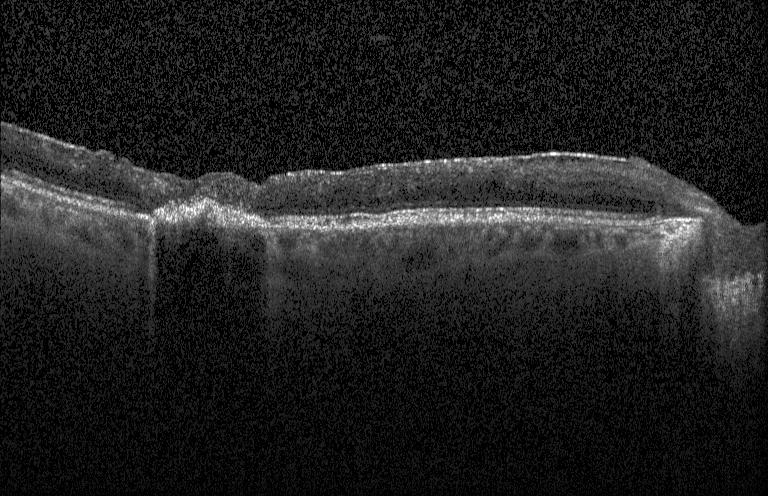 OCT line scan. Instrument: Heidelberg Spectralis — Assessment: a choroidal neovascular membrane.